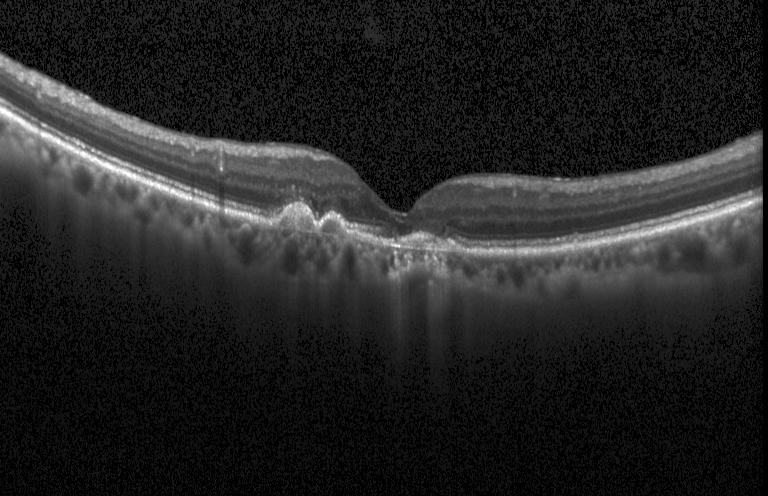

Through the macula · Heidelberg Spectralis · OCT line scan
Finding: a choroidal neovascular membrane.